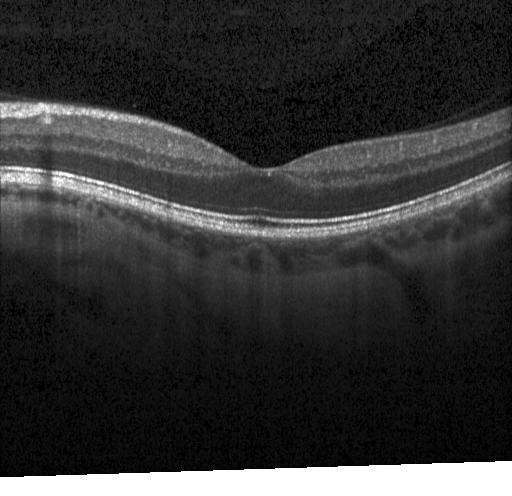

Finding: neither choroidal neovascularization, diabetic macular edema, nor drusen.